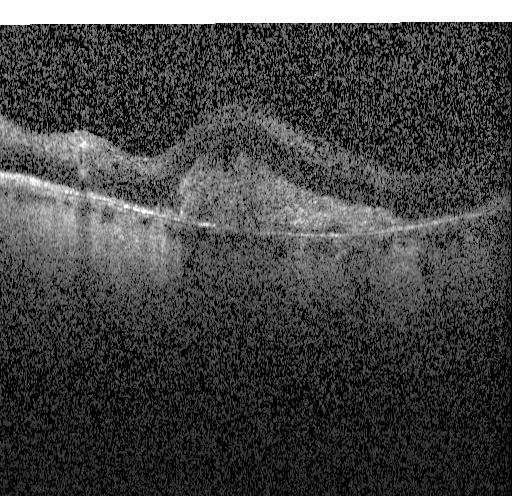 Finding: a choroidal neovascular membrane.